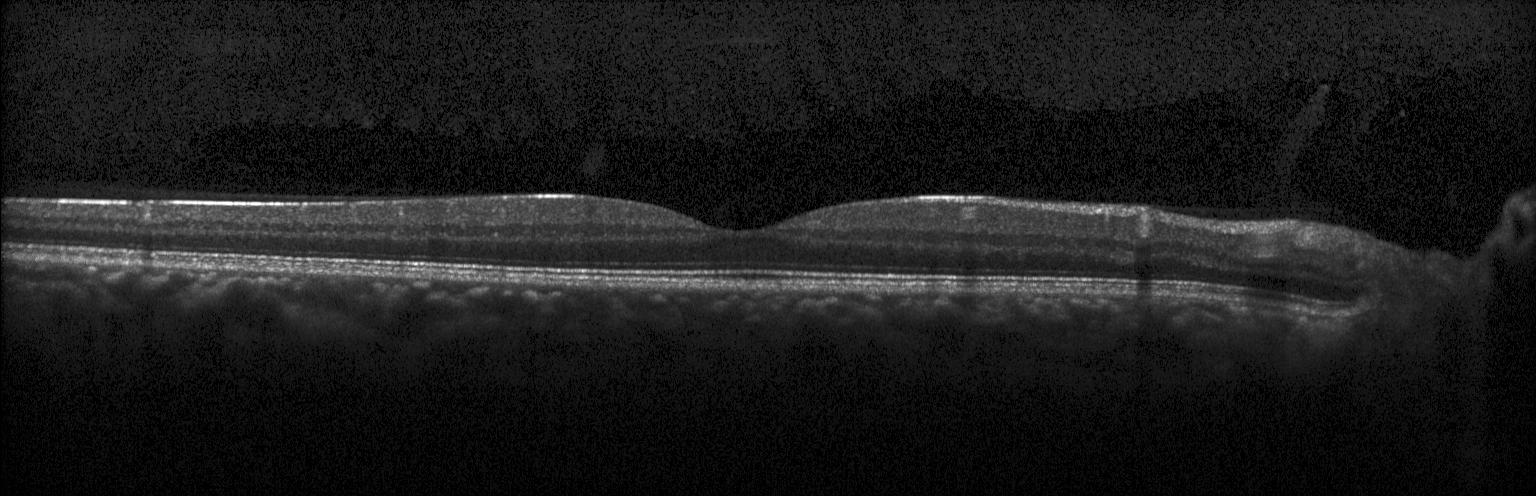

Heidelberg Spectralis. Optical coherence tomography scan — Macular OCT: no CNV, DME, or drusen.